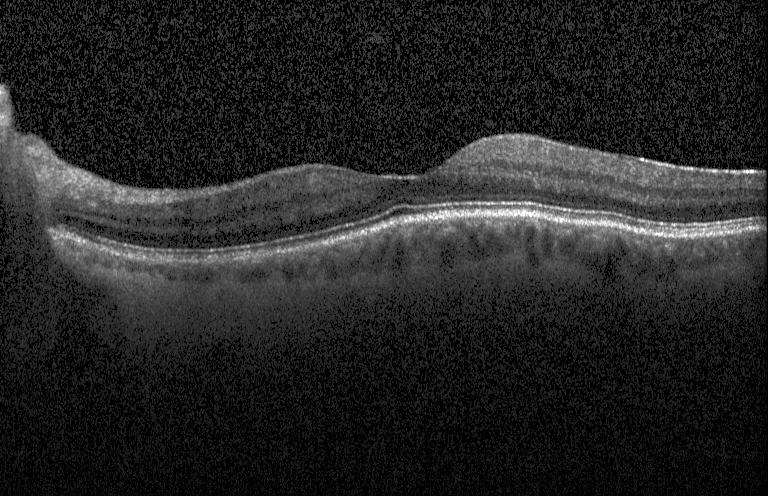 Heidelberg Spectralis OCT system; OCT B-scan
Diagnosis: no CNV, DME, or drusen.